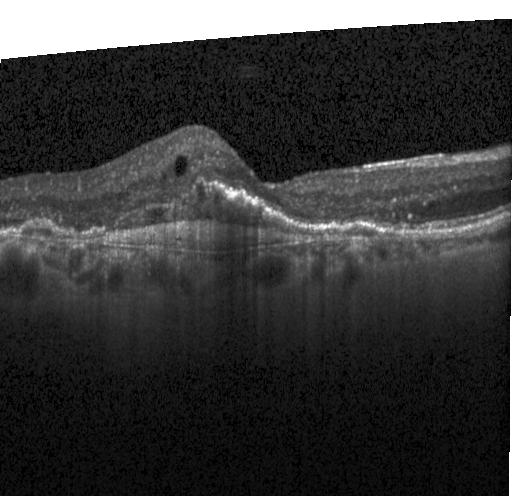

OCT B-scan · fovea-centered — Finding: a choroidal neovascular membrane.